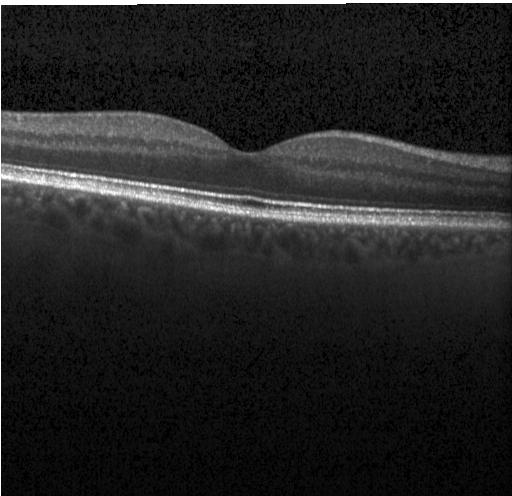

Heidelberg Spectralis OCT system · horizontal scan through the fovea · retinal OCT B-scan. Impression: neither choroidal neovascularization, diabetic macular edema, nor drusen.